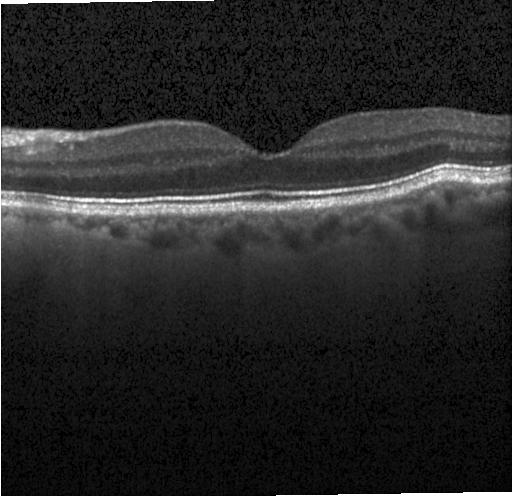

Heidelberg Spectralis; OCT B-scan; SD-OCT.
The scan shows no choroidal neovascularization, no diabetic macular edema, and no drusen.